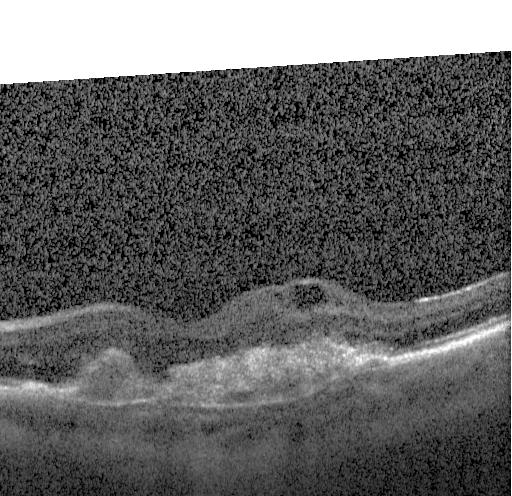

Impression: choroidal neovascularization (CNV).